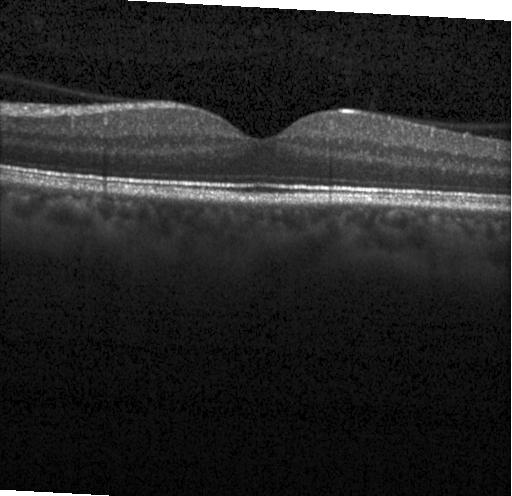 Macular OCT: no evidence of choroidal neovascularization, diabetic macular edema, or drusen.